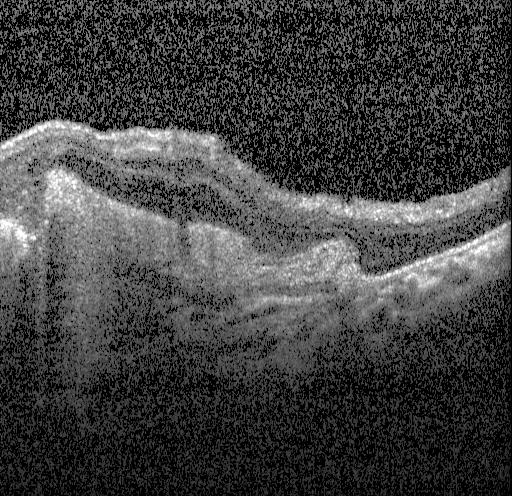
Finding: a choroidal neovascular membrane.